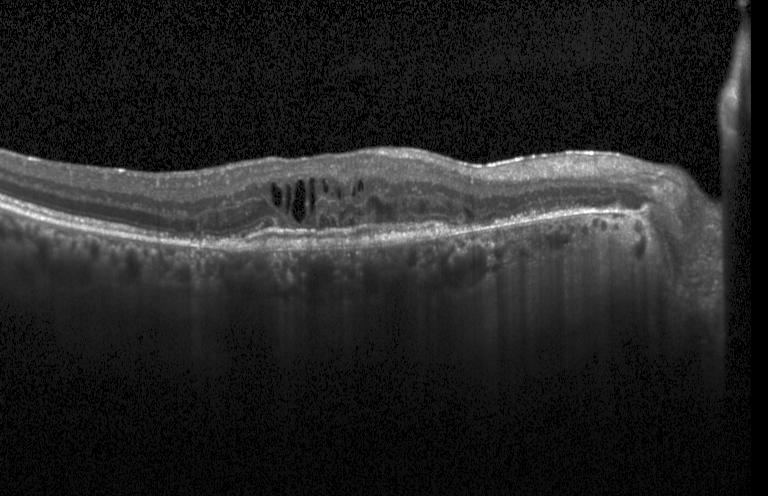

Spectral-domain OCT B-scan: choroidal neovascularization (CNV).